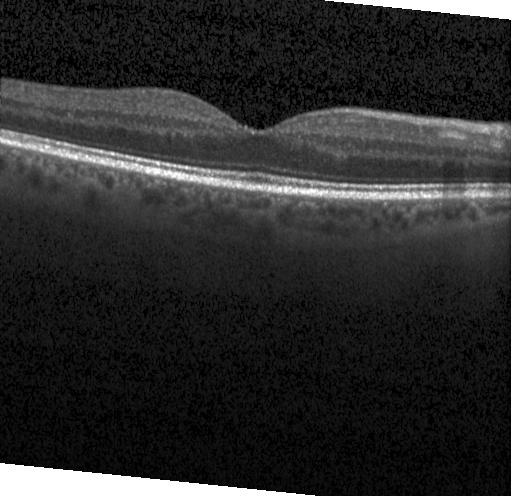 Heidelberg Spectralis OCT system. Optical coherence tomography scan. Fovea-centered. SD-OCT
Assessment: neither CNV, DME, nor drusen.